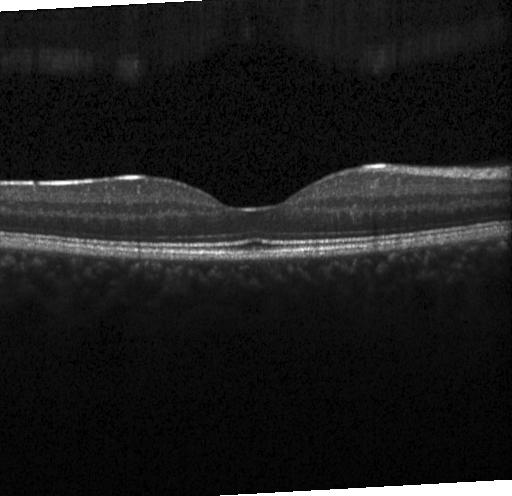
OCT line scan, centered on the fovea, spectral-domain OCT — Diagnosis: no evidence of choroidal neovascularization, diabetic macular edema, or drusen.